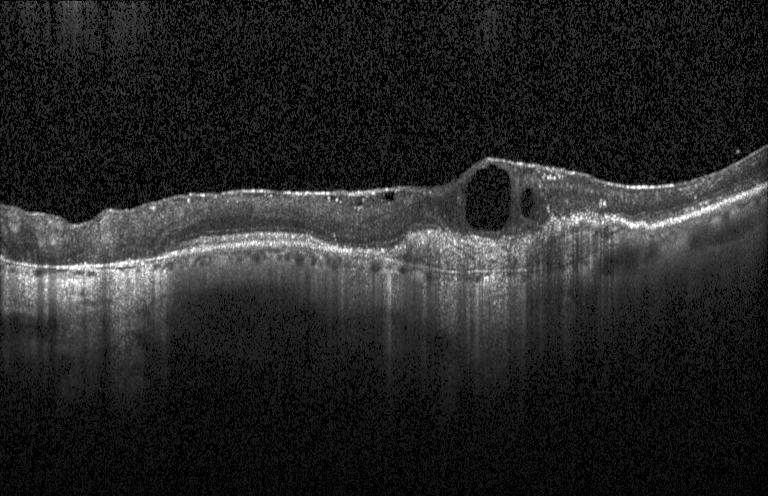

Retinal OCT B-scan, spectral-domain optical coherence tomography — Dx: a choroidal neovascular membrane.